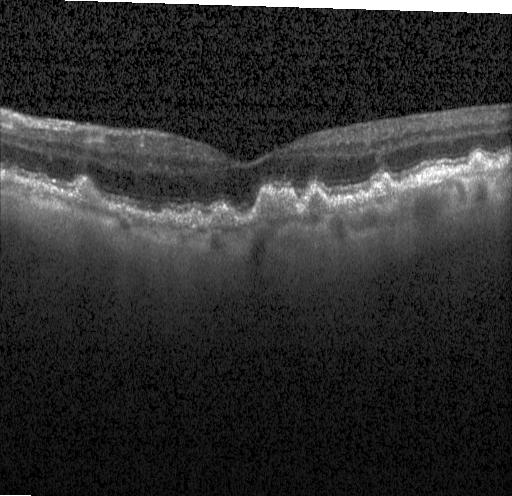 Retinal OCT B-scan · fovea-centered — Drusen.